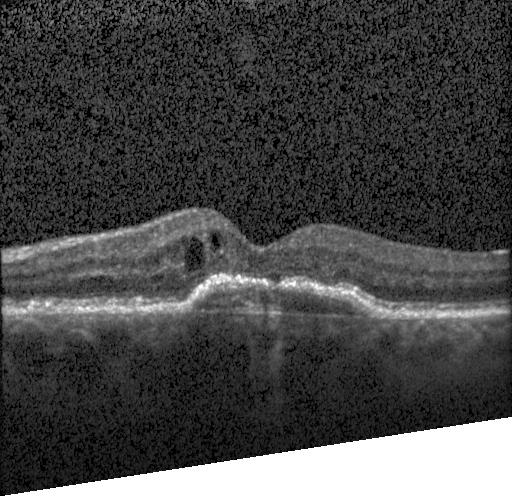
Impression: a choroidal neovascular membrane.